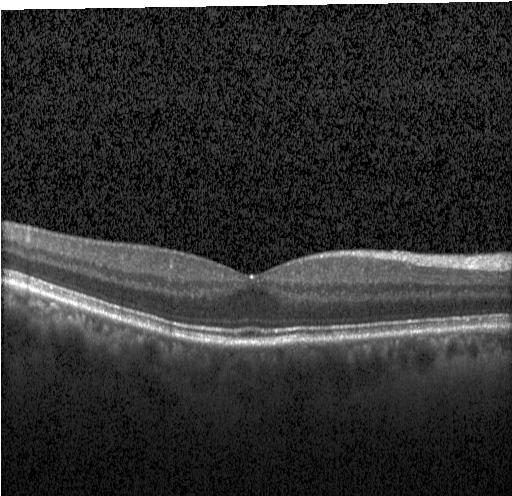 OCT B-scan; macular scan; Heidelberg Spectralis.
Impression: no choroidal neovascularization, diabetic macular edema, or drusen.